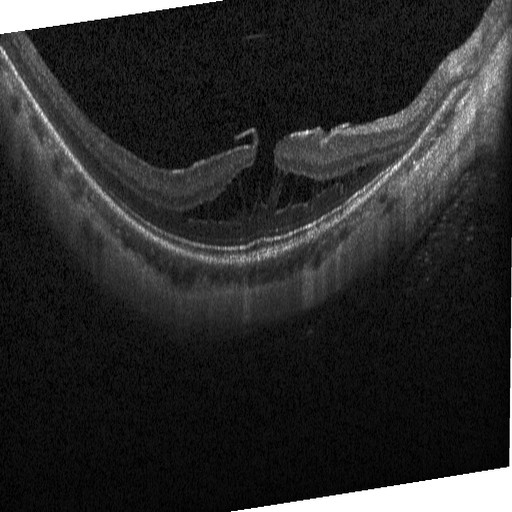 Finding: DME.